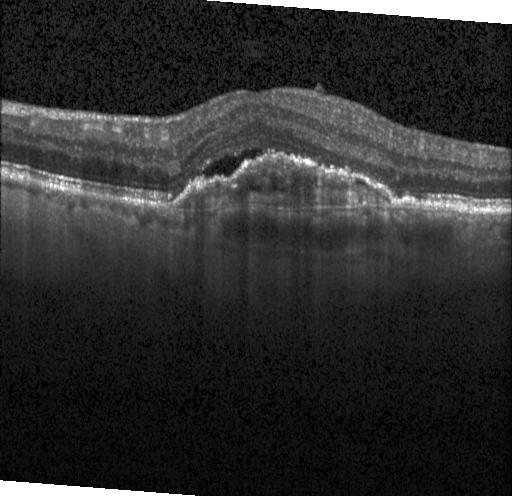
Horizontal scan through the fovea, instrument: Heidelberg Spectralis, OCT B-scan — Finding: a choroidal neovascular membrane.